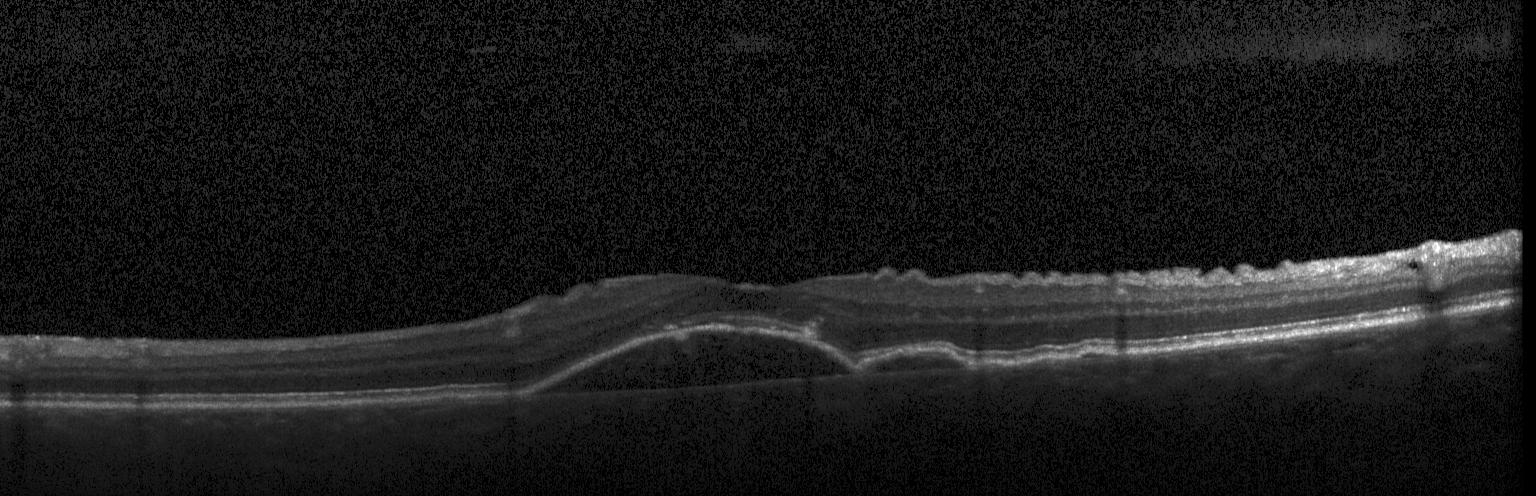 Finding: a choroidal neovascular membrane.